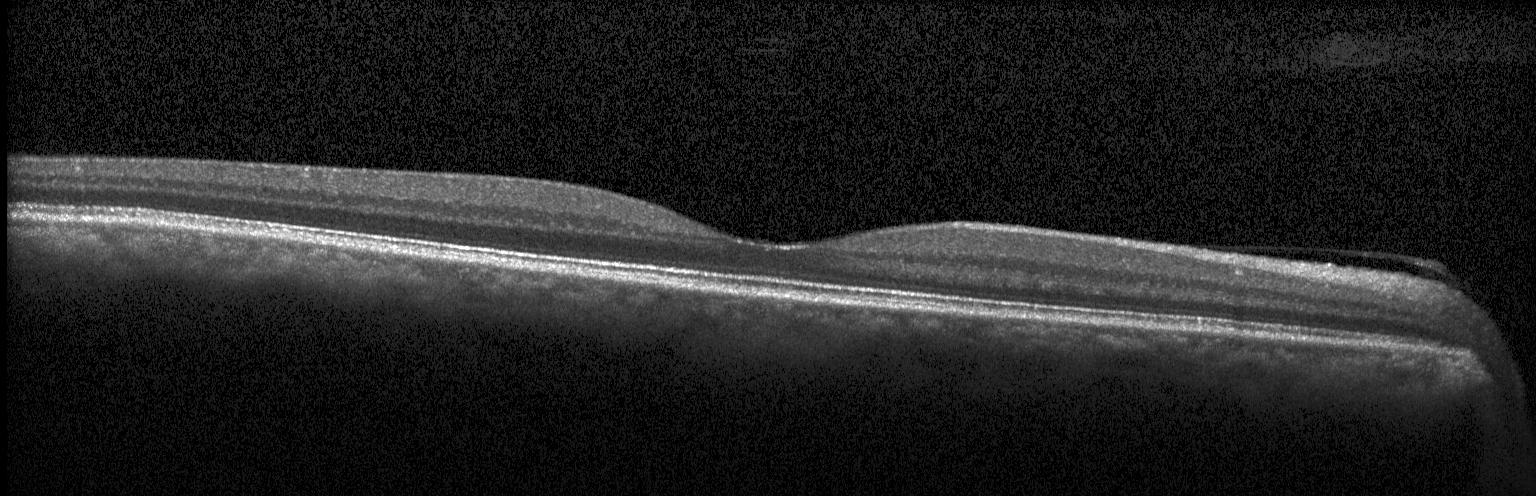

Fovea-centered · Heidelberg Spectralis OCT system · OCT B-scan.
Dx: neither choroidal neovascularization, diabetic macular edema, nor drusen.